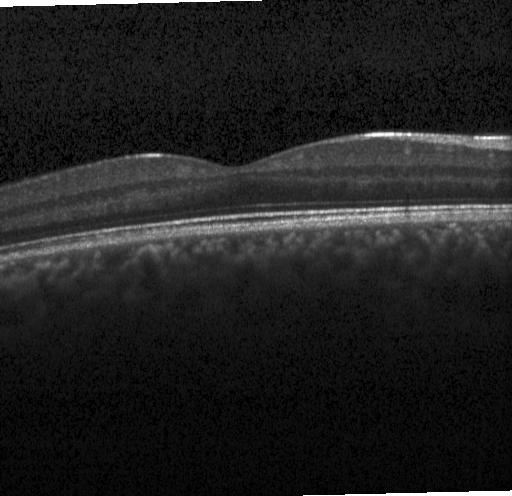

OCT line scan. Assessment: no CNV, DME, or drusen.